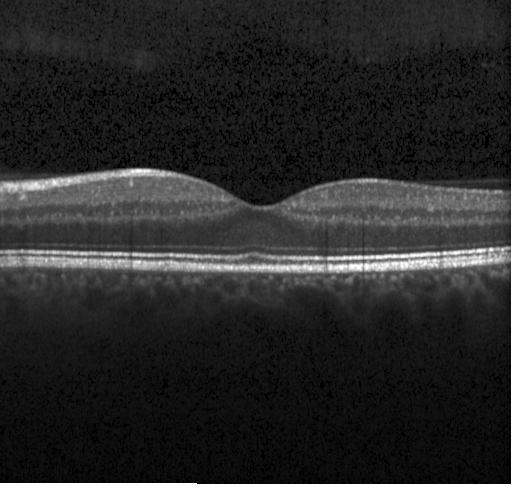 Impression: no evidence of choroidal neovascularization, diabetic macular edema, or drusen.